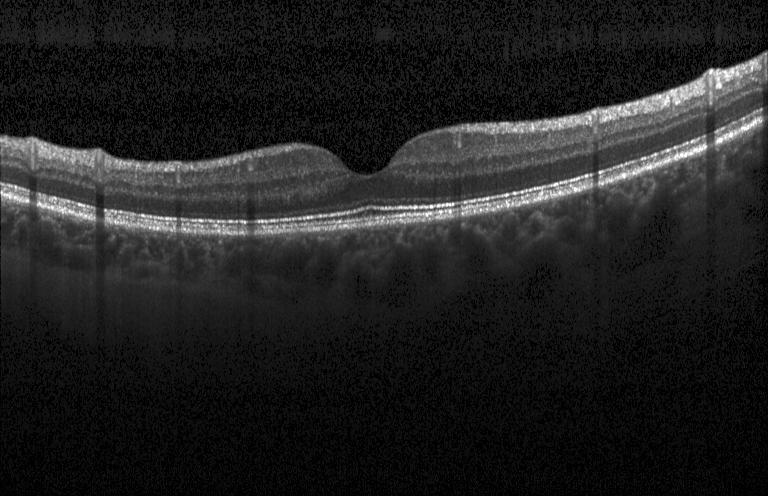 Retinal OCT B-scan. OCT finding: no choroidal neovascularization, no diabetic macular edema, and no drusen.